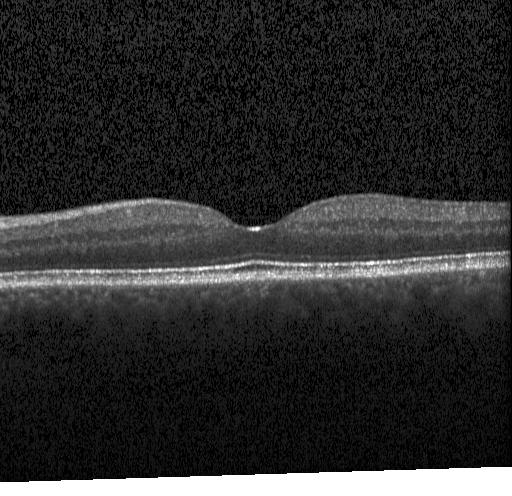
Macular OCT demonstrating neither choroidal neovascularization, diabetic macular edema, nor drusen.